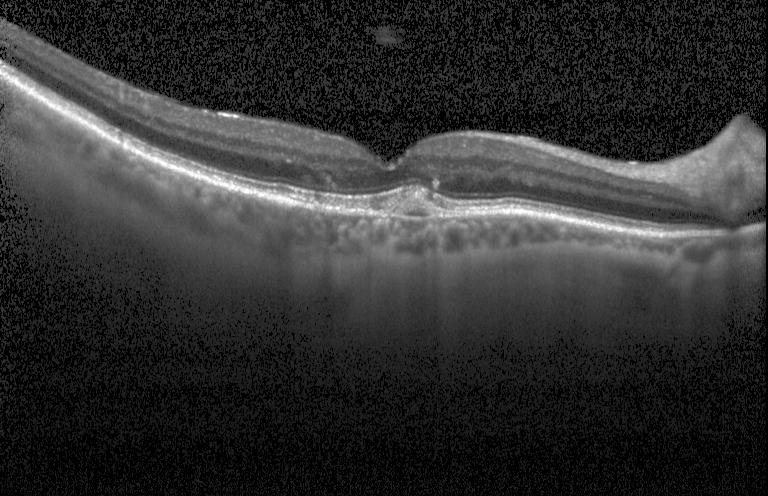 Macular OCT demonstrating a choroidal neovascular membrane.